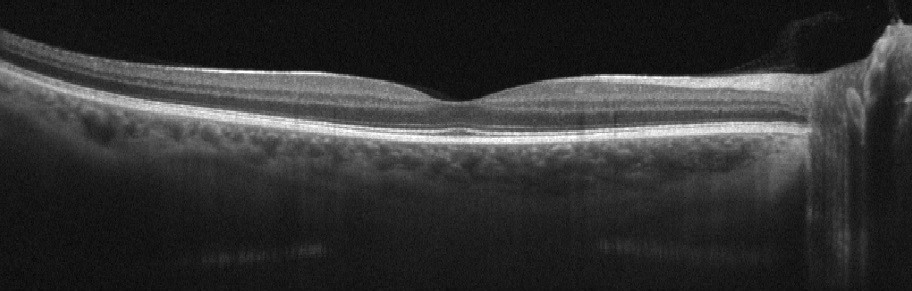 Diagnosis: no evidence of AMD, DME, ERM, RAO, RVO, or VID.